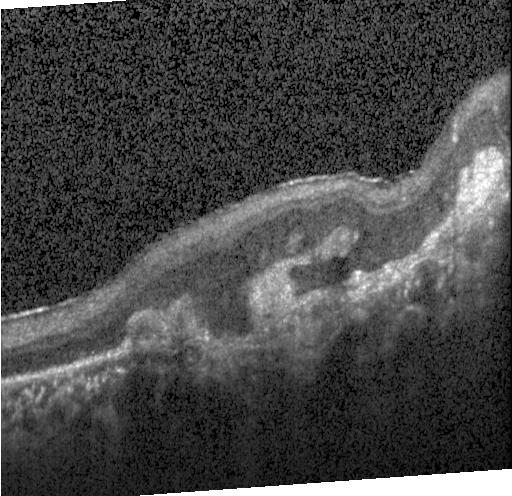

OCT B-scan. Acquired on a Heidelberg Spectralis. SD-OCT
Finding: a choroidal neovascular membrane.